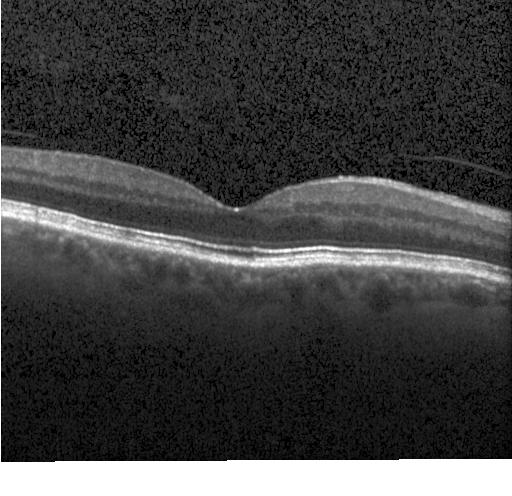
Heidelberg Spectralis; macular scan; optical coherence tomography B-scan; SD-OCT. OCT finding: no evidence of CNV, DME, or drusen.